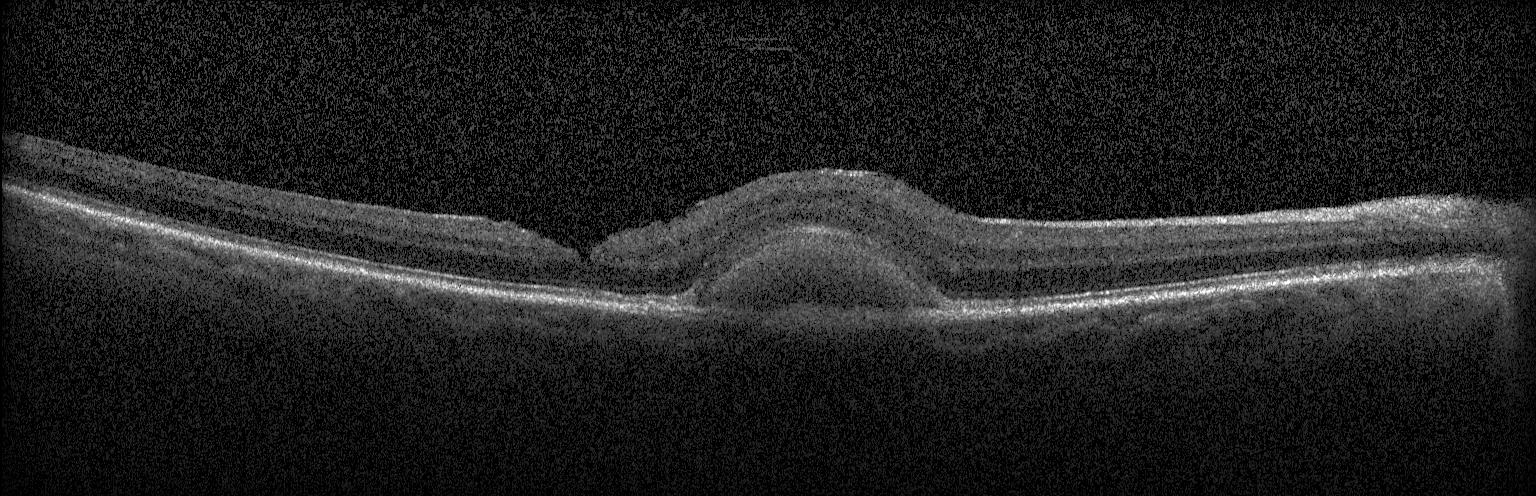 Diagnosis: a choroidal neovascular membrane.